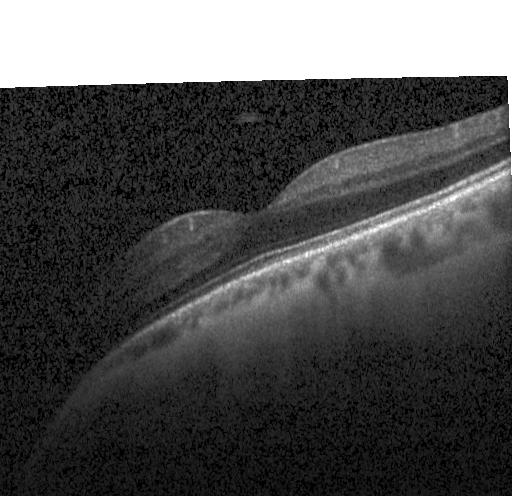 Macular scan · OCT B-scan. Impression: no evidence of choroidal neovascularization, diabetic macular edema, or drusen.